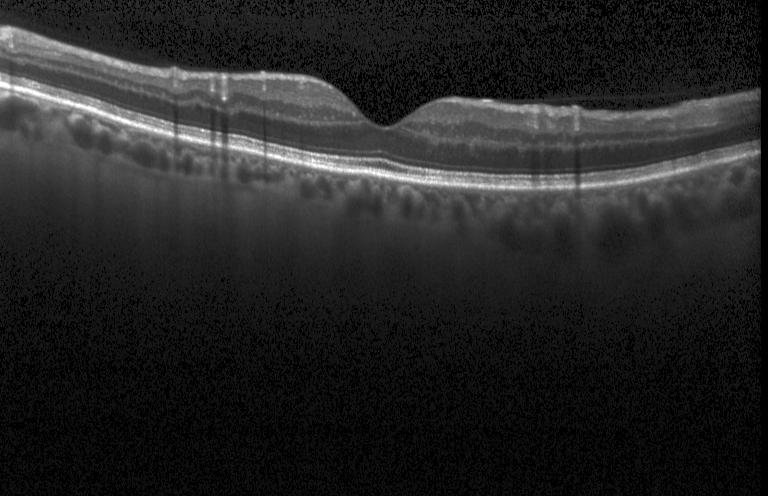 Heidelberg Spectralis OCT system, OCT B-scan. OCT finding: neither CNV, DME, nor drusen.